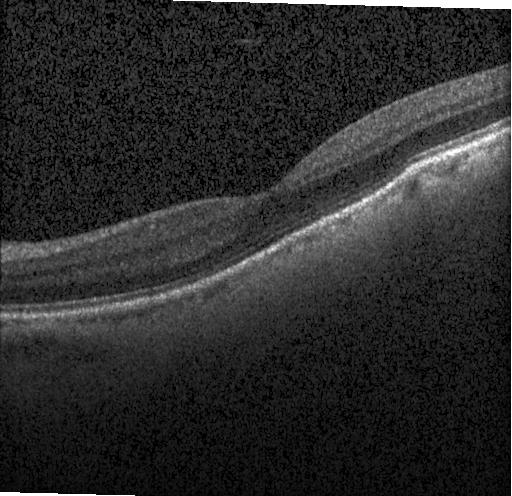 Optical coherence tomography scan · centered on the fovea.
The scan shows no evidence of choroidal neovascularization, diabetic macular edema, or drusen.